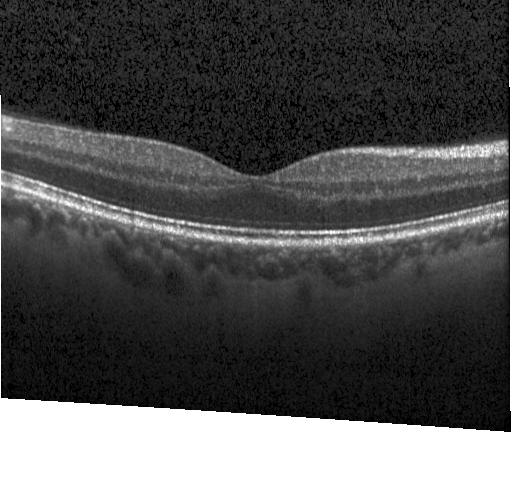 Retinal OCT B-scan. SD-OCT. Heidelberg Spectralis OCT system. Finding: no evidence of choroidal neovascularization, diabetic macular edema, or drusen.